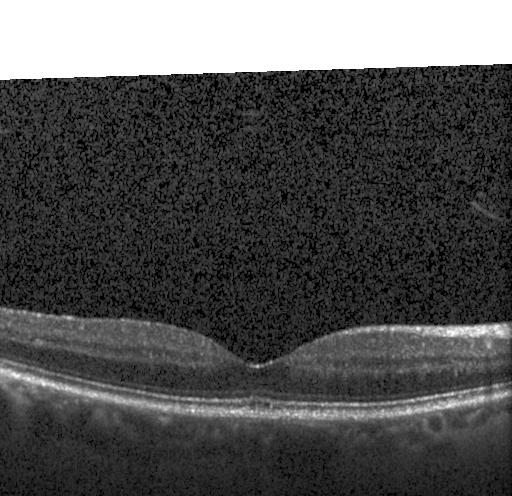 OCT finding: neither CNV, DME, nor drusen.